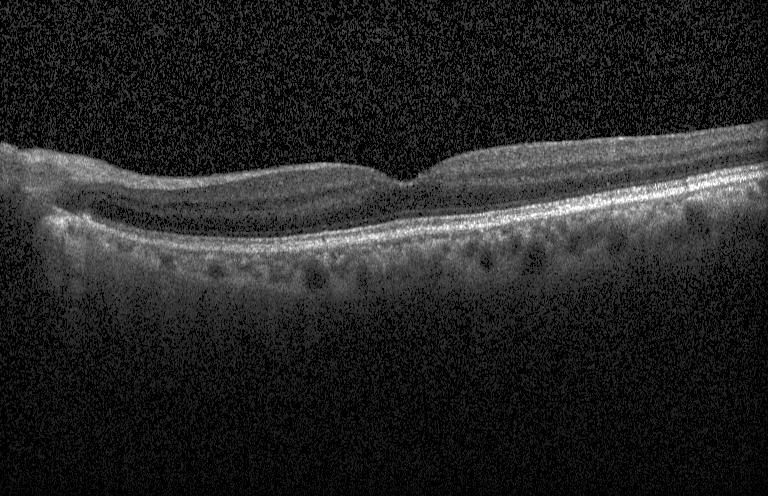
Optical coherence tomography scan. Dx: neither choroidal neovascularization, diabetic macular edema, nor drusen.